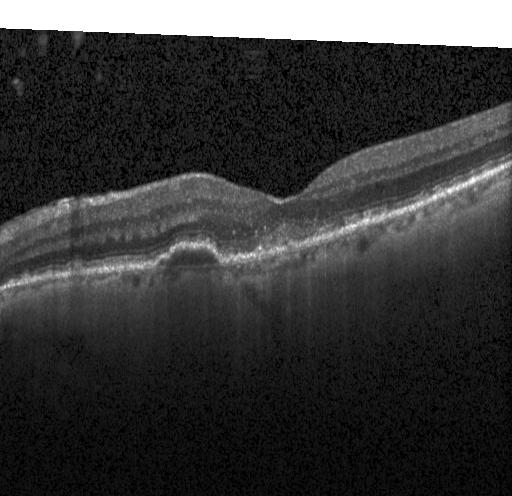 Impression: a choroidal neovascular membrane.